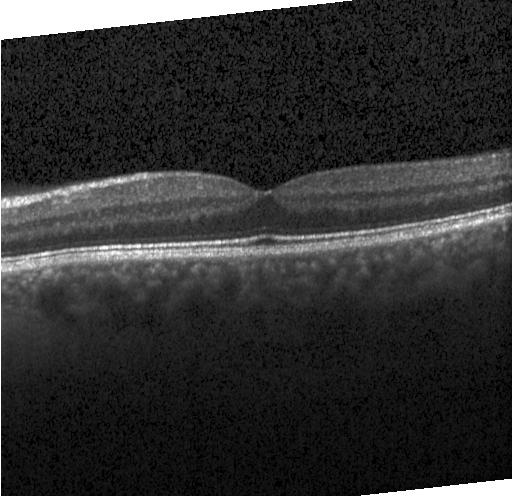

Horizontal scan through the fovea. Retinal OCT cross-section. Spectral-domain optical coherence tomography.
Macular OCT: no evidence of CNV, DME, or drusen.